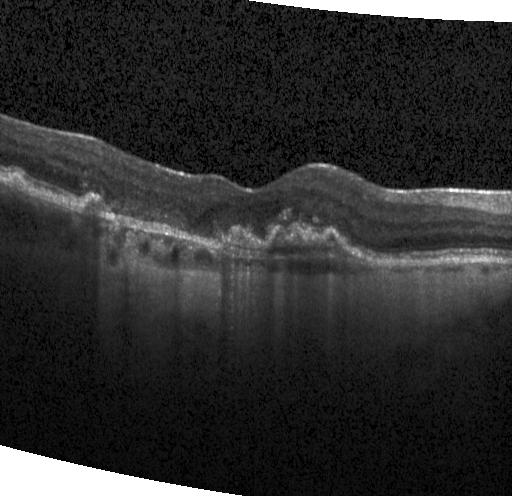 OCT finding: a choroidal neovascular membrane.